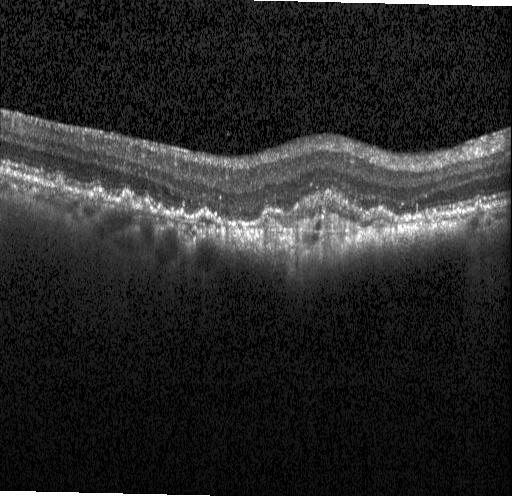

Optical coherence tomography scan · spectral-domain OCT
OCT finding: a choroidal neovascular membrane.